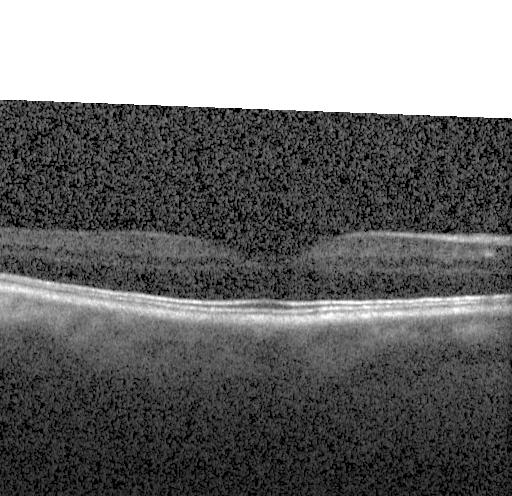

Diagnosis: no choroidal neovascularization, diabetic macular edema, or drusen.